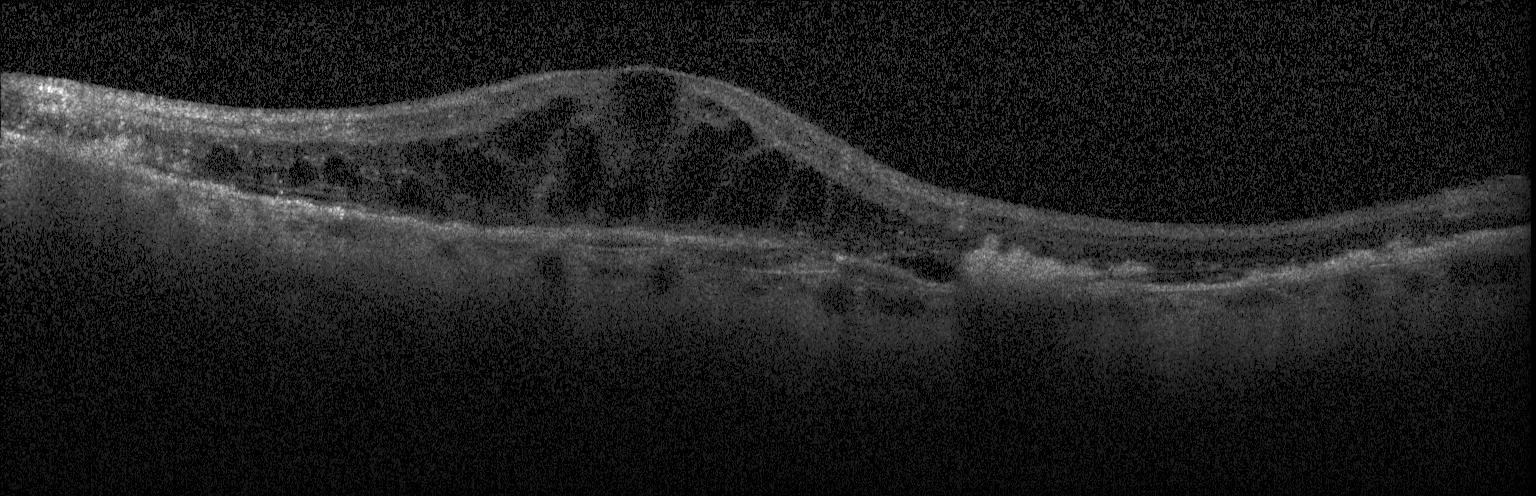

SD-OCT. OCT line scan. Centered on the fovea
Diagnosis: CNV.